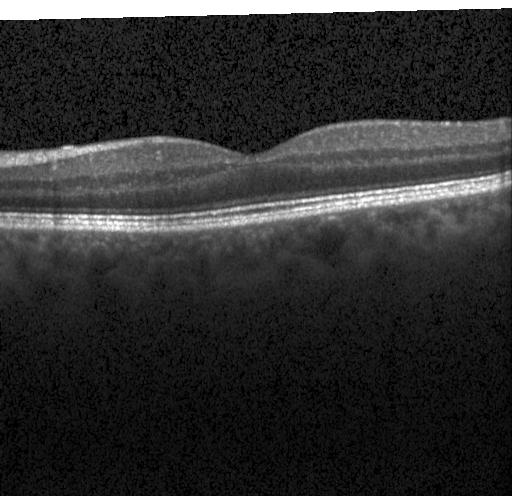
Optical coherence tomography scan — Macular OCT: no choroidal neovascularization, no diabetic macular edema, and no drusen.